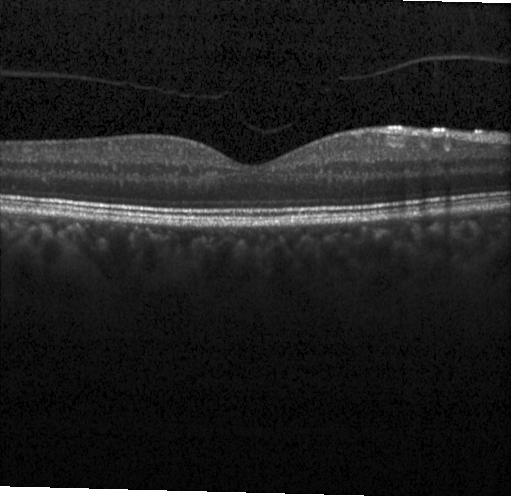
OCT line scan, SD-OCT, horizontal scan through the fovea. Diagnosis: no choroidal neovascularization, diabetic macular edema, or drusen.